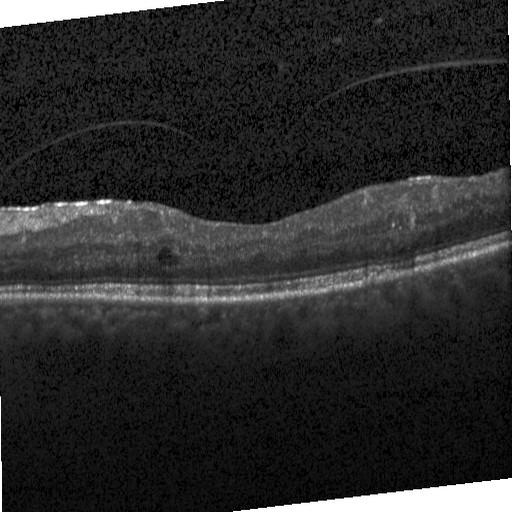

Assessment: diabetic macular edema.